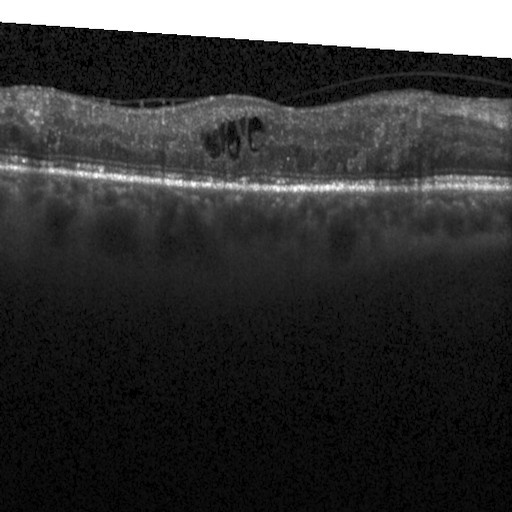

OCT line scan. Heidelberg Spectralis OCT system. Impression: diabetic macular edema (DME).